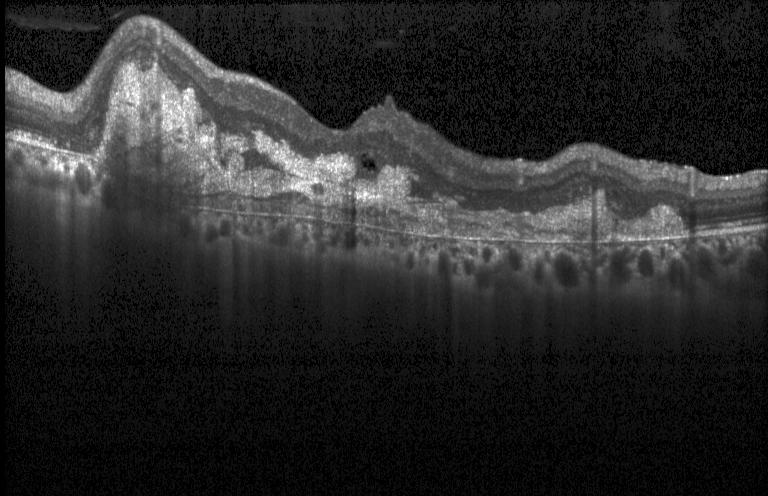

Spectral-domain optical coherence tomography, retinal OCT B-scan.
CNV.